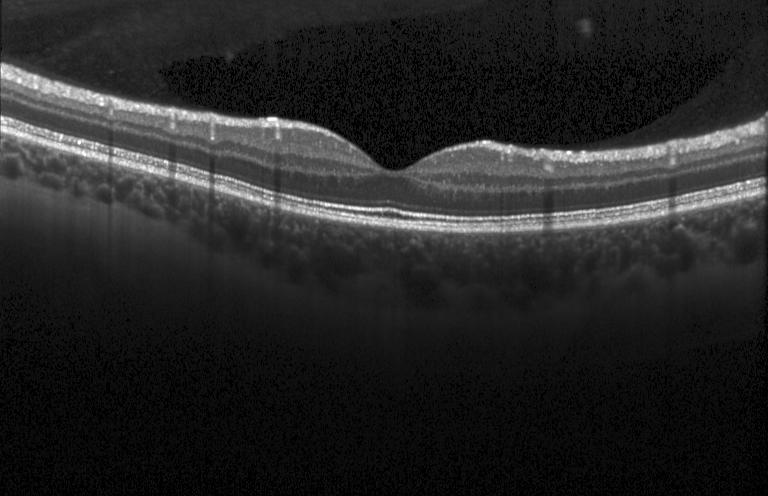 Retinal OCT B-scan · fovea-centered · spectral-domain optical coherence tomography. Macular OCT: no evidence of choroidal neovascularization, diabetic macular edema, or drusen.